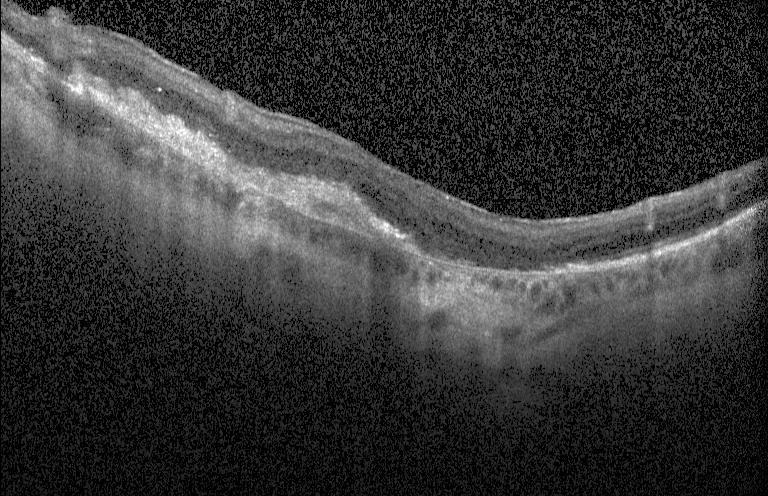
Finding: choroidal neovascularization.